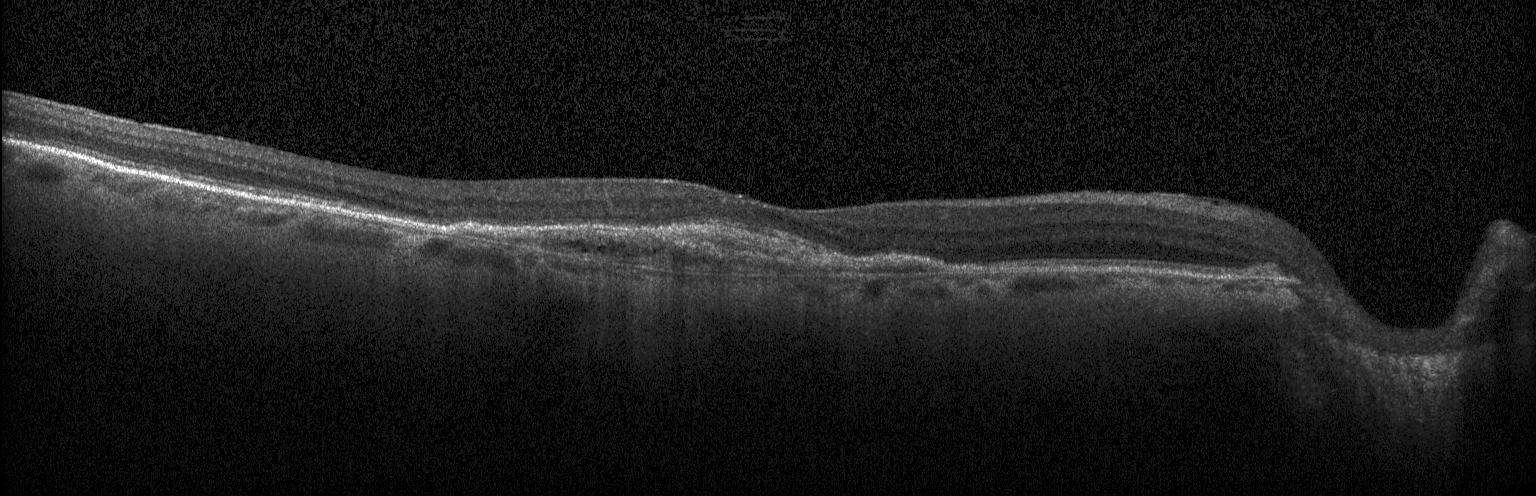
Spectral-domain optical coherence tomography, optical coherence tomography B-scan, horizontal scan through the fovea.
This B-scan demonstrates a choroidal neovascular membrane.